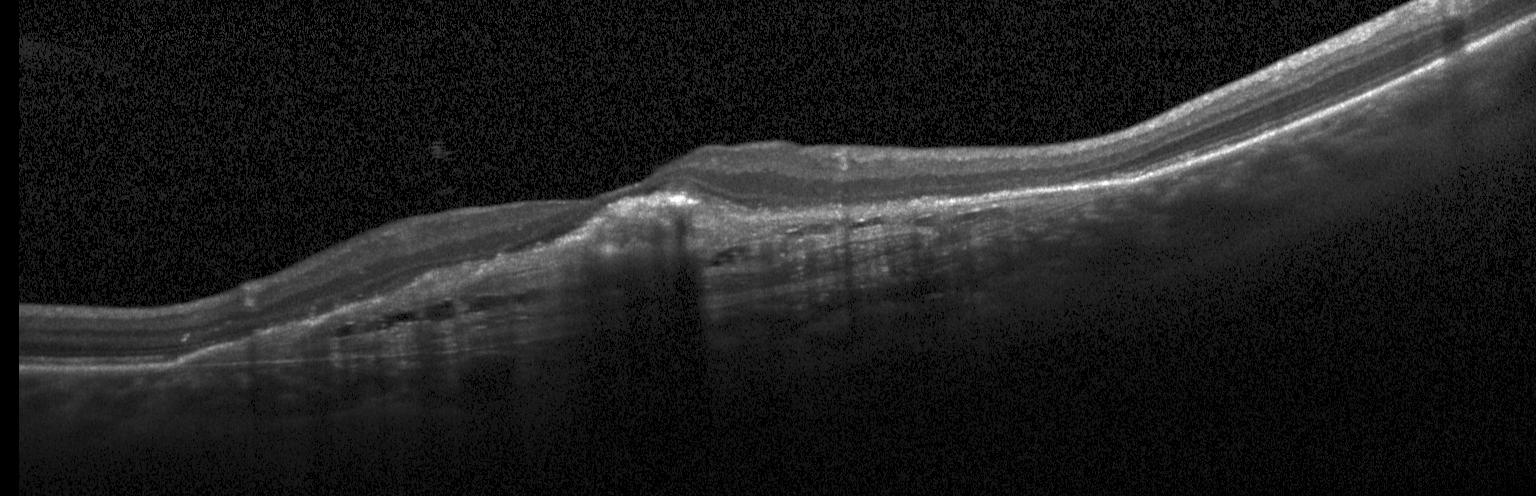

The scan shows choroidal neovascularization.